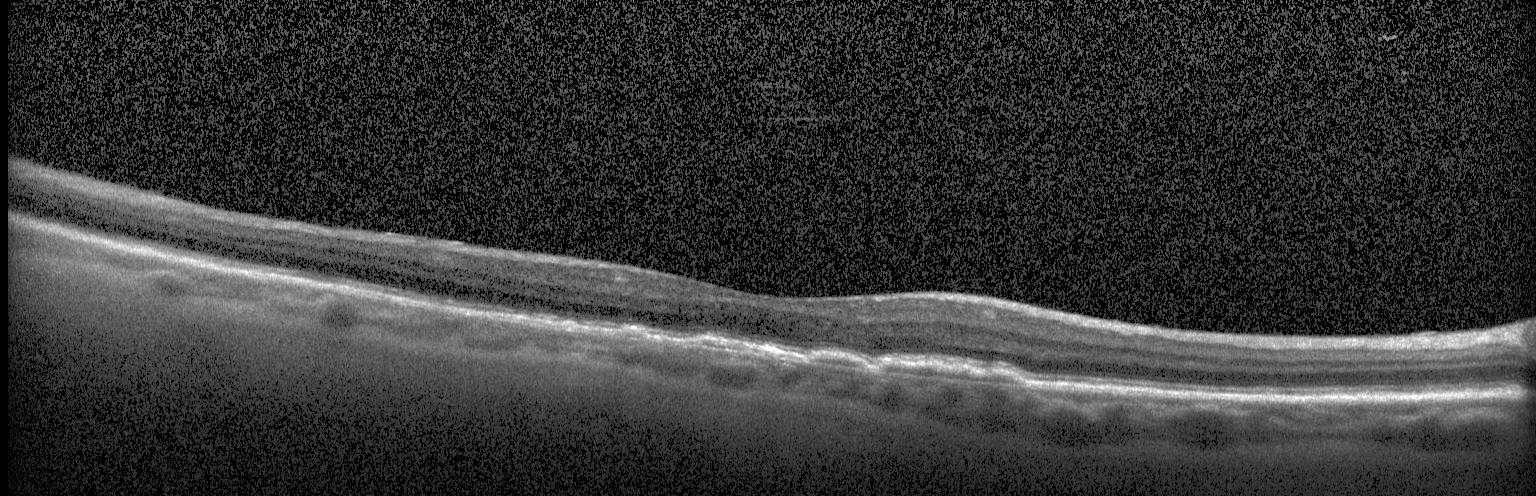 Optical coherence tomography scan
OCT finding: a choroidal neovascular membrane.